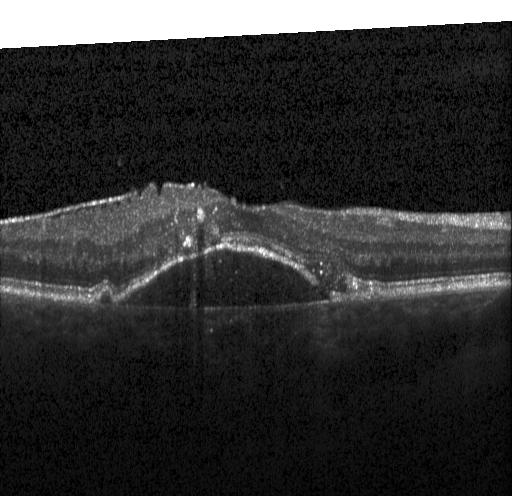

OCT line scan · horizontal scan through the fovea. Finding: a choroidal neovascular membrane.